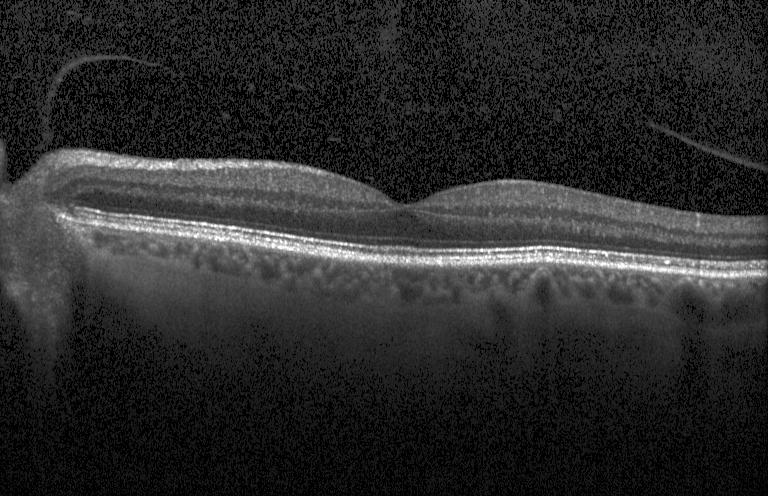 Heidelberg Spectralis OCT system, retinal OCT B-scan
OCT finding: no choroidal neovascularization, diabetic macular edema, or drusen.